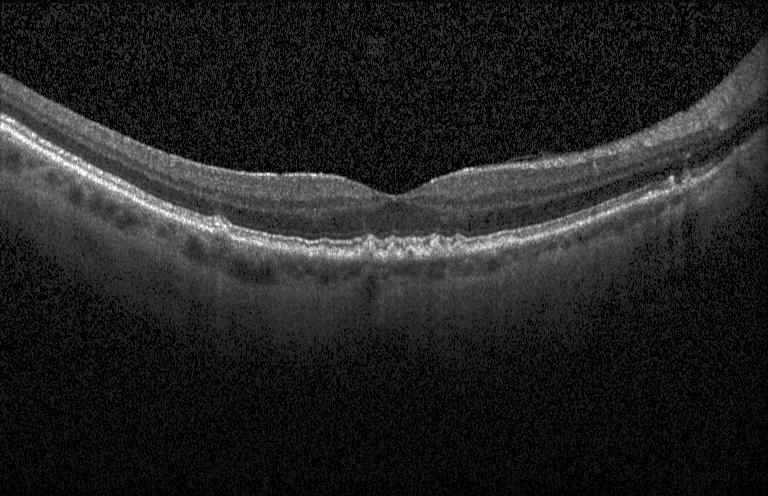
OCT line scan — Impression: multiple drusen.